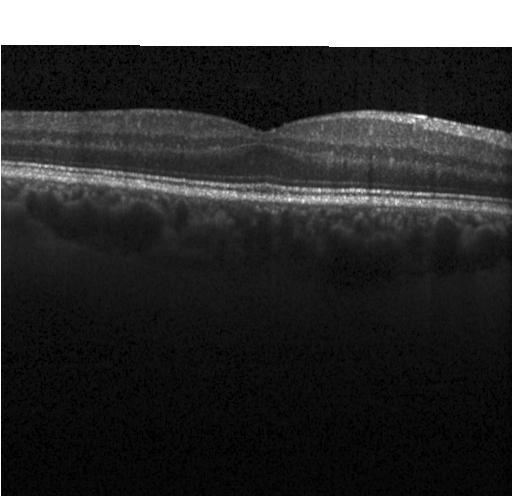 Retinal OCT cross-section. Finding: no CNV, no DME, and no drusen.